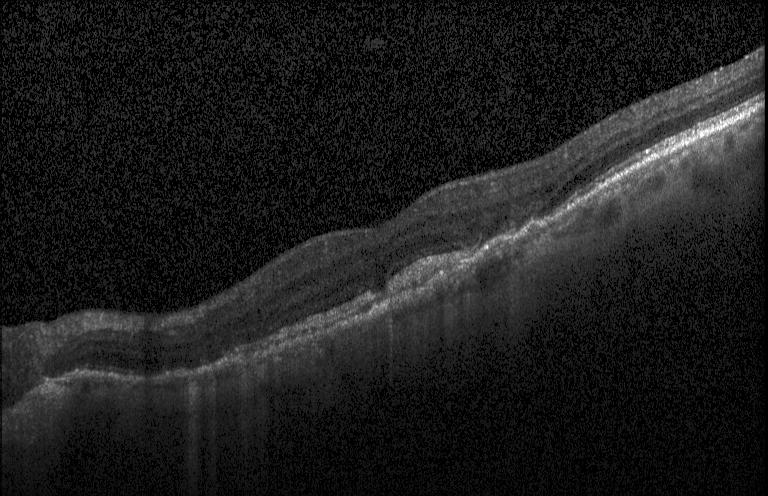
Retinal OCT B-scan — This B-scan demonstrates choroidal neovascularization.